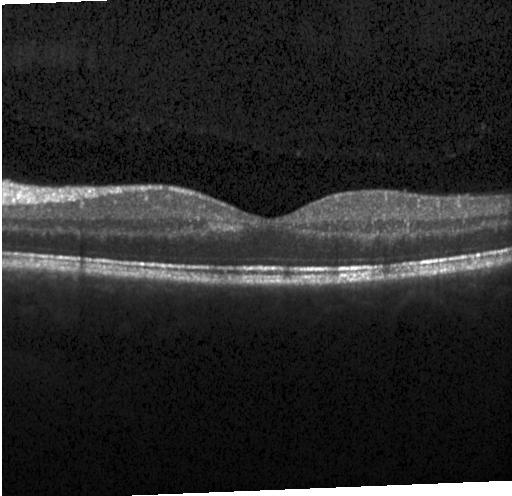 Optical coherence tomography B-scan. Acquired on a Heidelberg Spectralis. Spectral-domain OCT. OCT finding: no evidence of choroidal neovascularization, diabetic macular edema, or drusen.